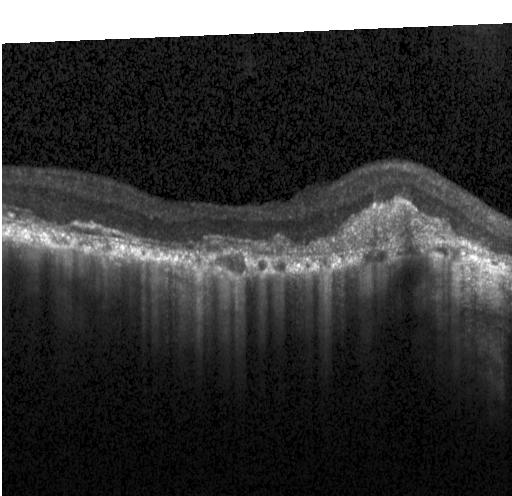
Retinal OCT B-scan. Spectral-domain OCT
Impression: CNV.